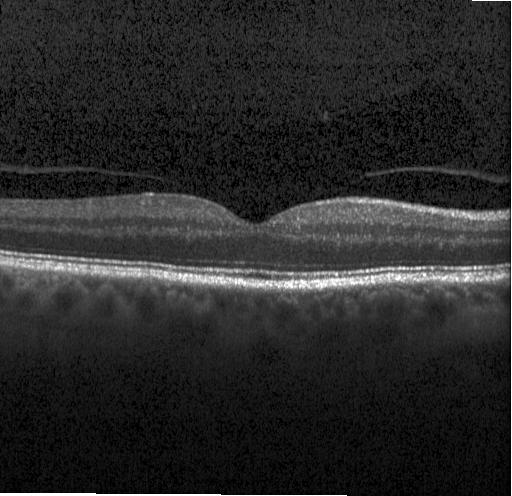
Heidelberg Spectralis · macular scan · OCT B-scan · spectral-domain OCT. Impression: no choroidal neovascularization, diabetic macular edema, or drusen.